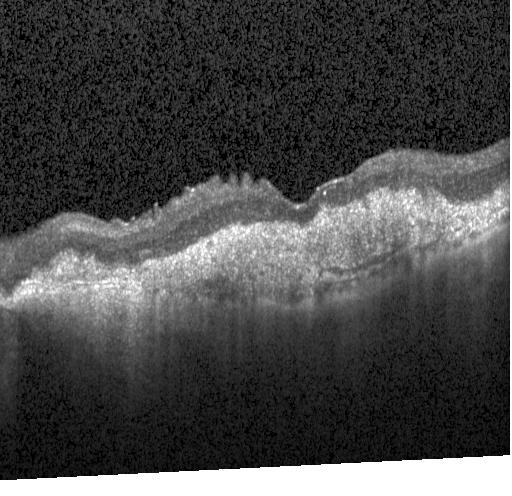

Diagnosis: a choroidal neovascular membrane.